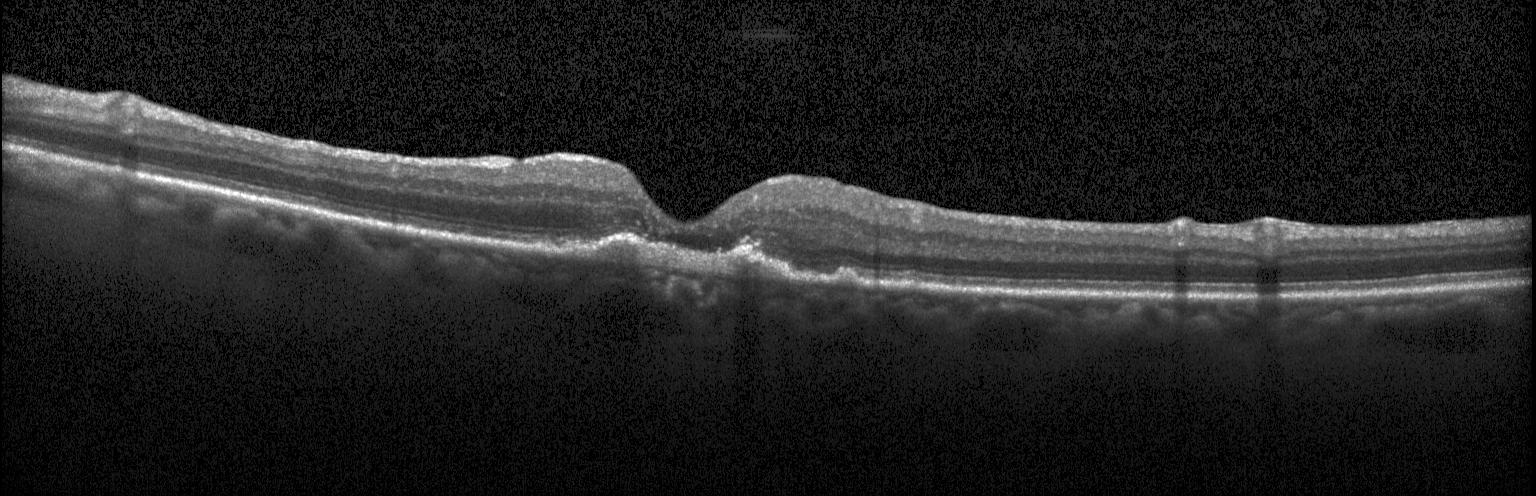
Optical coherence tomography B-scan. A choroidal neovascular membrane.